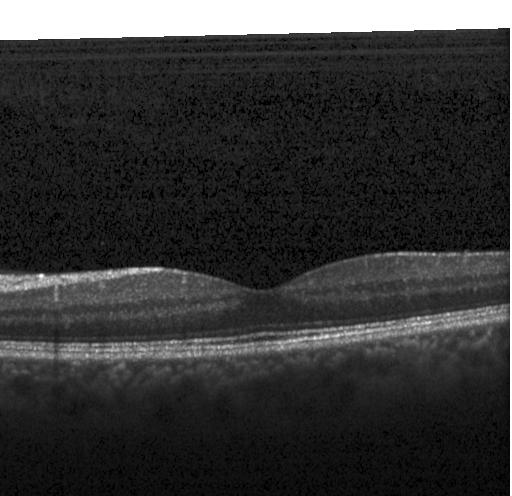

Optical coherence tomography B-scan; SD-OCT; through the macula.
Macular OCT: no choroidal neovascularization, diabetic macular edema, or drusen.